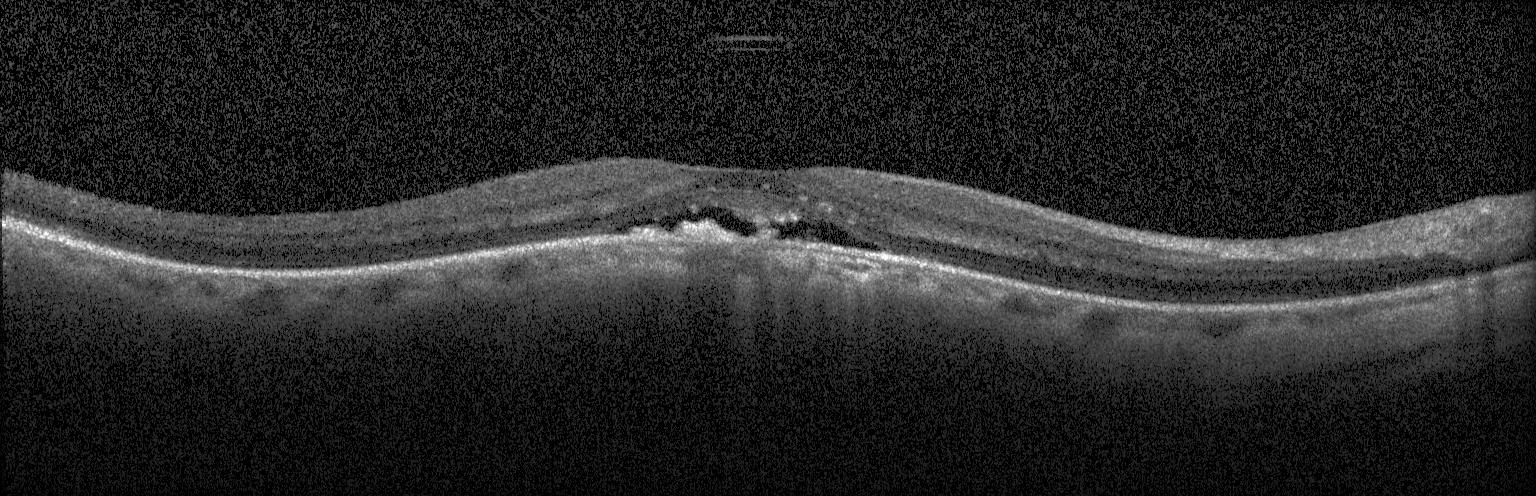

Centered on the fovea · retinal OCT B-scan. Diagnosis: a choroidal neovascular membrane.